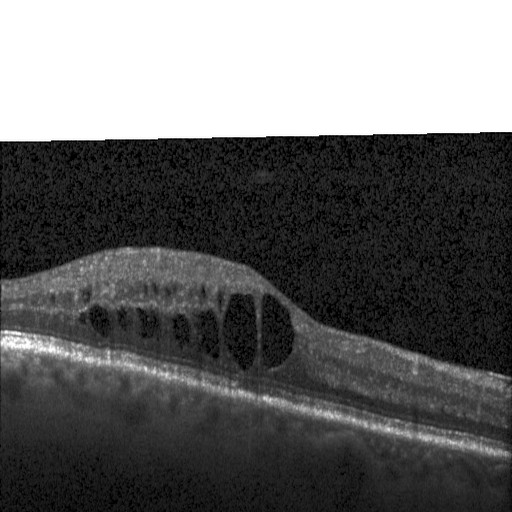 OCT scan showing DME.